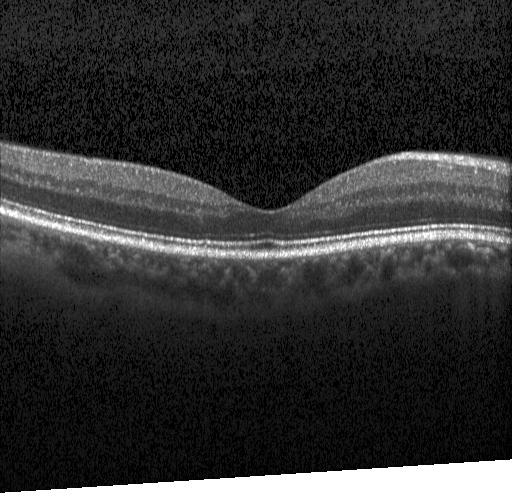 Impression: no evidence of CNV, DME, or drusen.